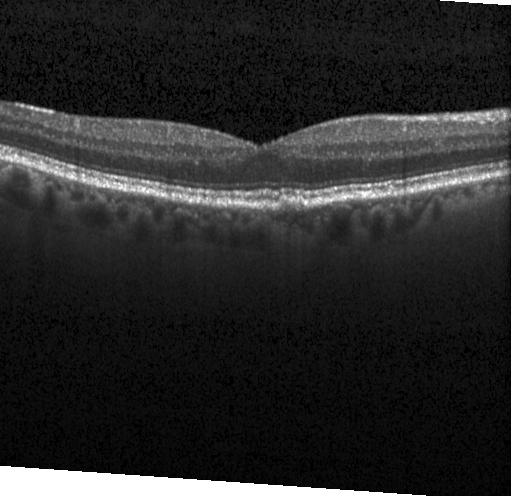
Heidelberg Spectralis OCT system. Spectral-domain optical coherence tomography. Macular scan. Optical coherence tomography scan
Finding: multiple drusen.